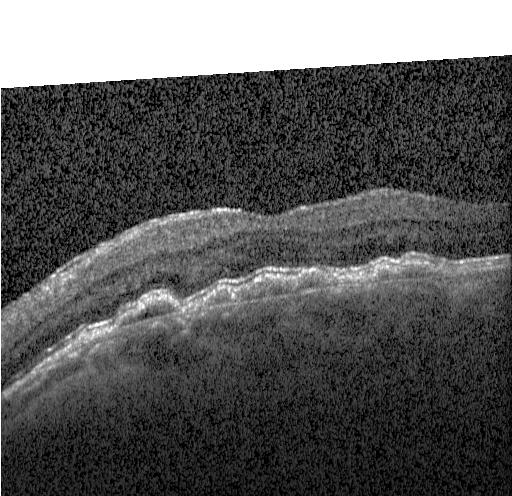 Heidelberg Spectralis OCT system, retinal OCT cross-section, SD-OCT, fovea-centered
Diagnosis: choroidal neovascularization.